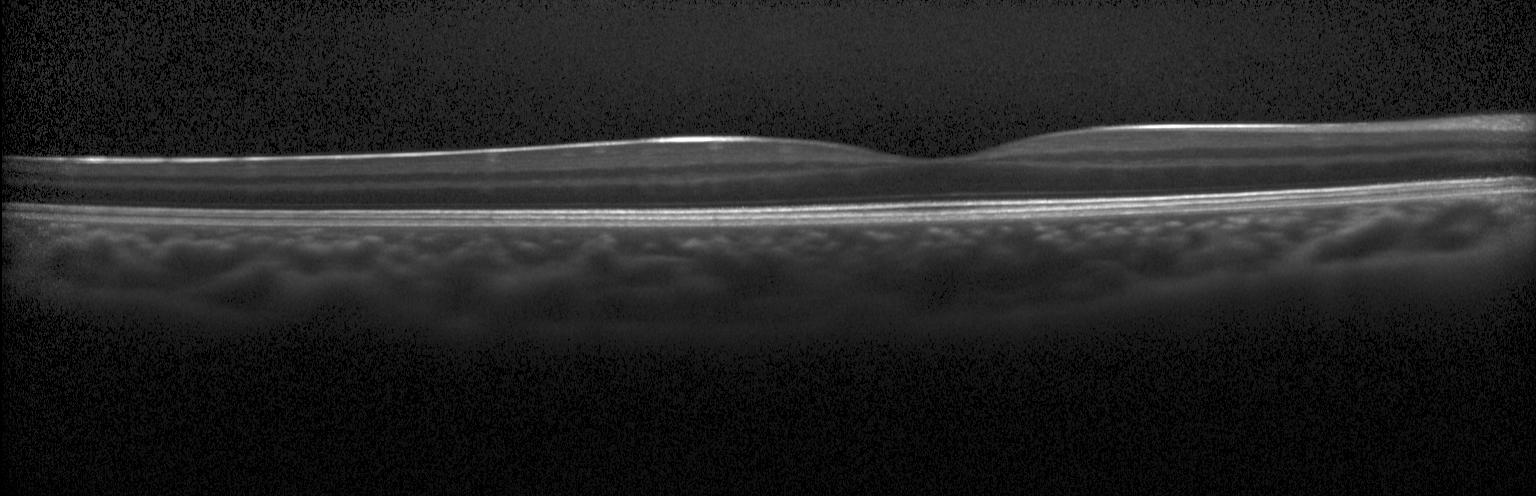
Instrument: Heidelberg Spectralis, centered on the fovea, retinal OCT B-scan, spectral-domain optical coherence tomography — No choroidal neovascularization, diabetic macular edema, or drusen.